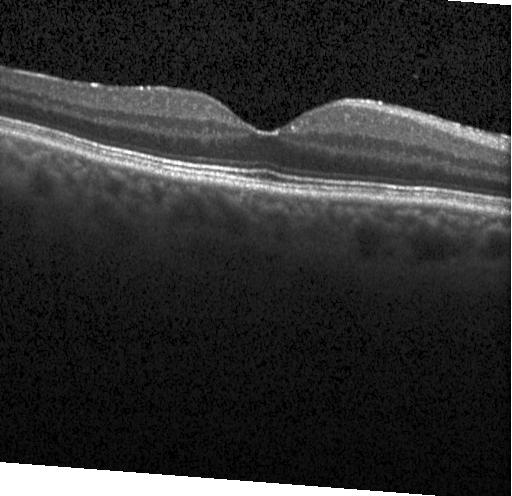

Retinal OCT cross-section showing neither CNV, DME, nor drusen.